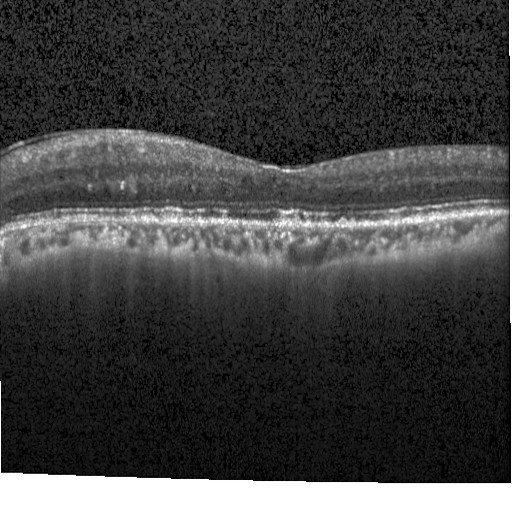 Instrument: Heidelberg Spectralis; spectral-domain optical coherence tomography; centered on the fovea; optical coherence tomography B-scan
This B-scan demonstrates DME.